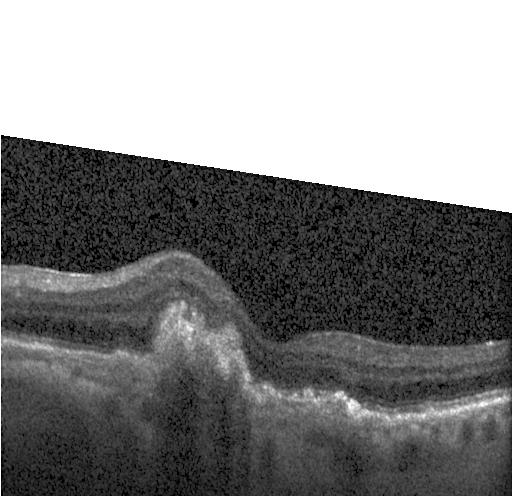

Retinal OCT cross-section, spectral-domain OCT, instrument: Heidelberg Spectralis
Impression: a choroidal neovascular membrane.